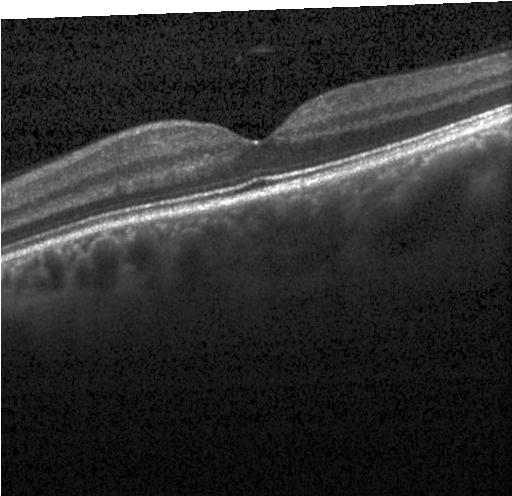 OCT B-scan; Heidelberg Spectralis OCT system
Finding: no choroidal neovascularization, no diabetic macular edema, and no drusen.